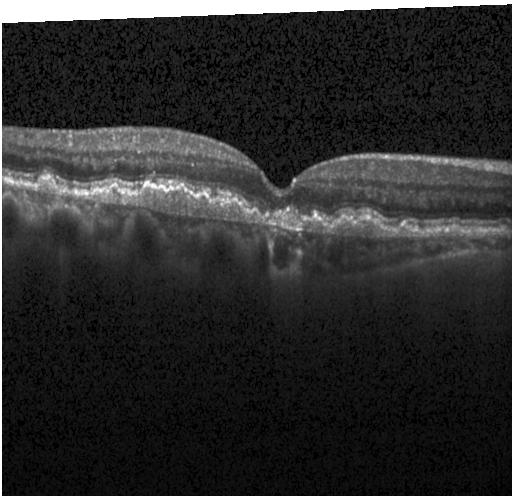 OCT B-scan. Heidelberg Spectralis. Spectral-domain optical coherence tomography. Centered on the fovea.
Impression: choroidal neovascularization.